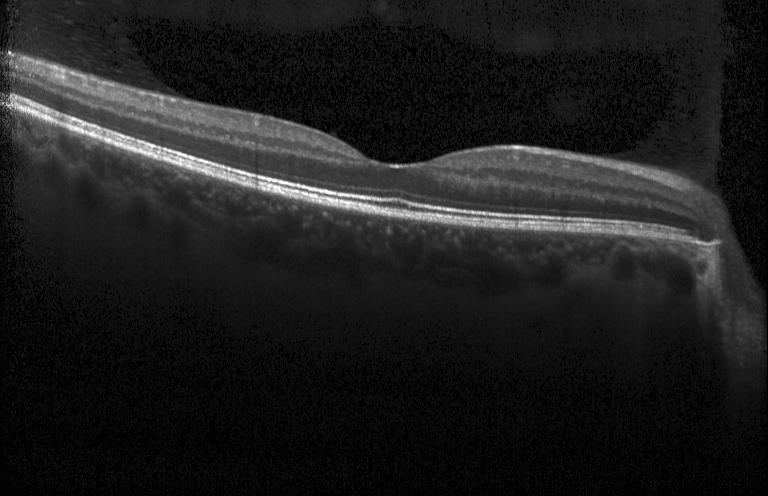 Optical coherence tomography scan; instrument: Heidelberg Spectralis.
The scan shows no choroidal neovascularization, diabetic macular edema, or drusen.